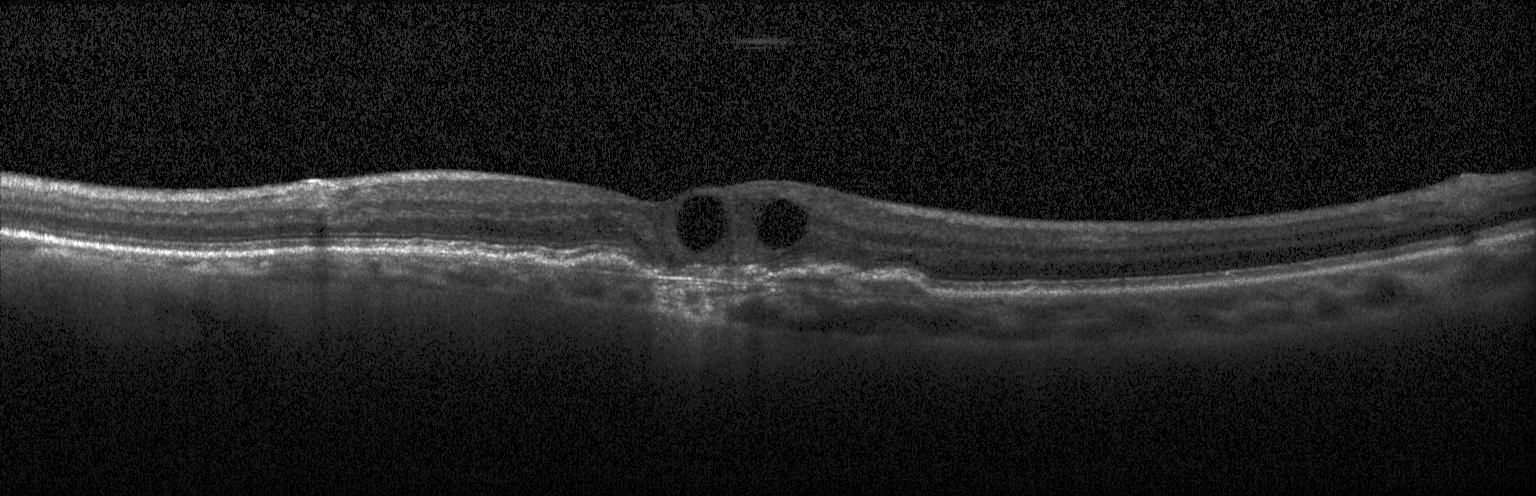

Dx: choroidal neovascularization.